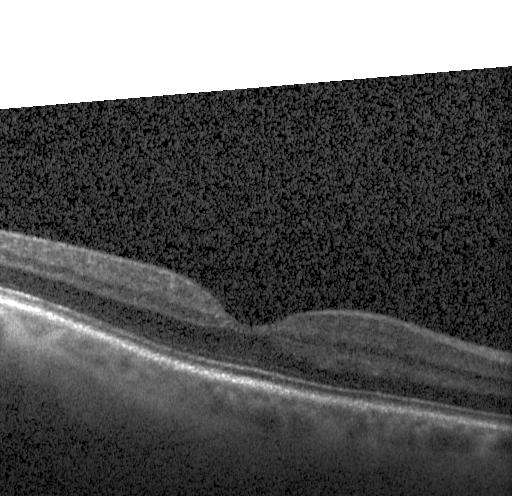
Instrument: Heidelberg Spectralis; retinal OCT cross-section — Finding: neither choroidal neovascularization, diabetic macular edema, nor drusen.